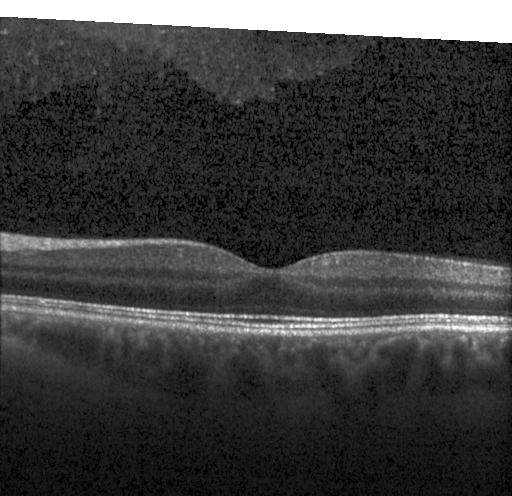
Impression: no evidence of choroidal neovascularization, diabetic macular edema, or drusen.